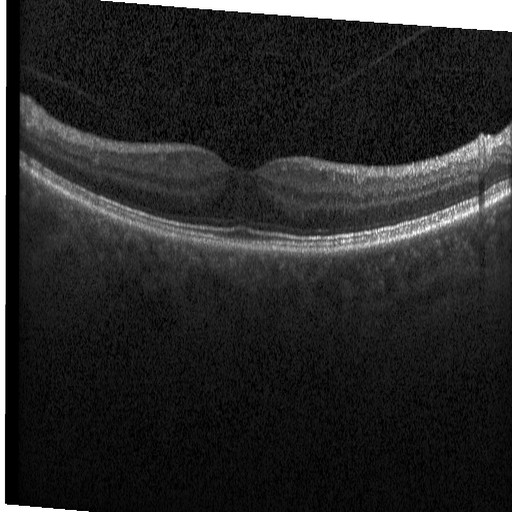 Instrument: Heidelberg Spectralis. Retinal OCT B-scan. Spectral-domain OCT. Centered on the fovea
Finding: DME.